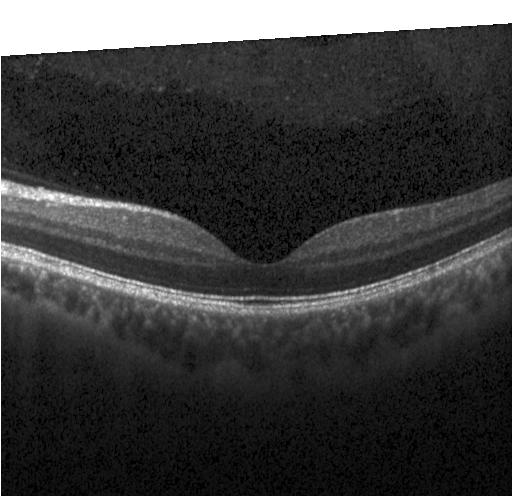
SD-OCT, retinal OCT B-scan — No choroidal neovascularization, no diabetic macular edema, and no drusen.